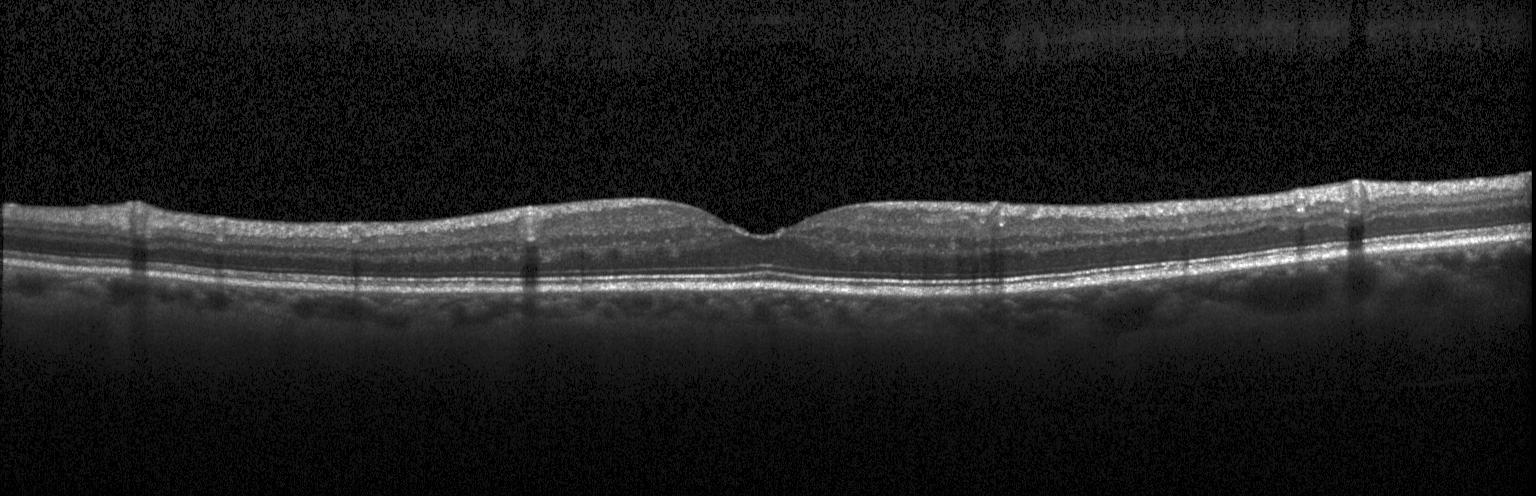 Optical coherence tomography scan; spectral-domain optical coherence tomography; acquired on a Heidelberg Spectralis
This B-scan demonstrates no CNV, DME, or drusen.